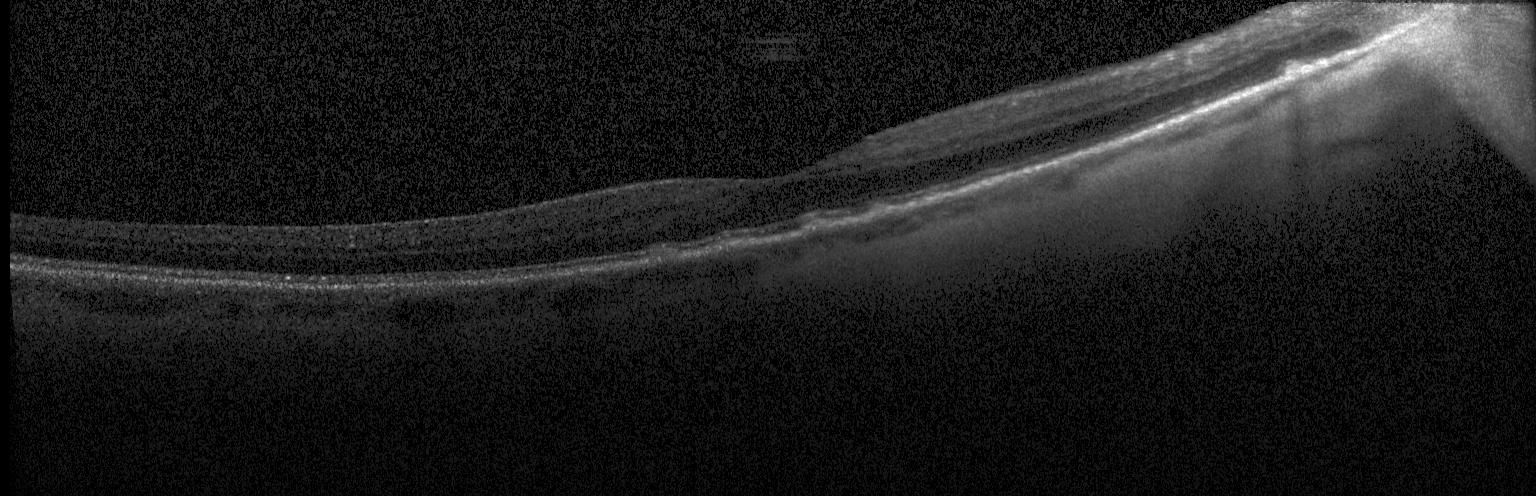

OCT scan showing drusen.